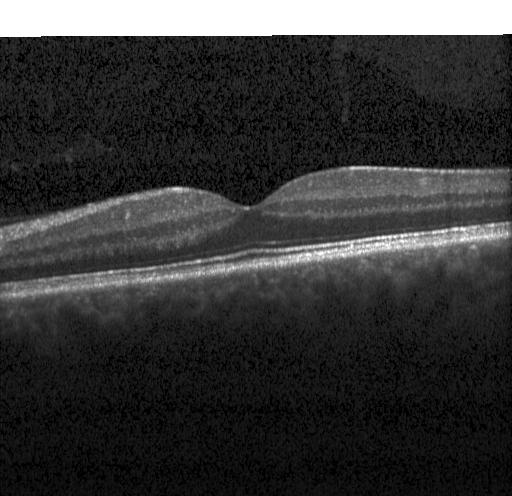
Retinal OCT cross-section · spectral-domain OCT.
Macular OCT: neither choroidal neovascularization, diabetic macular edema, nor drusen.